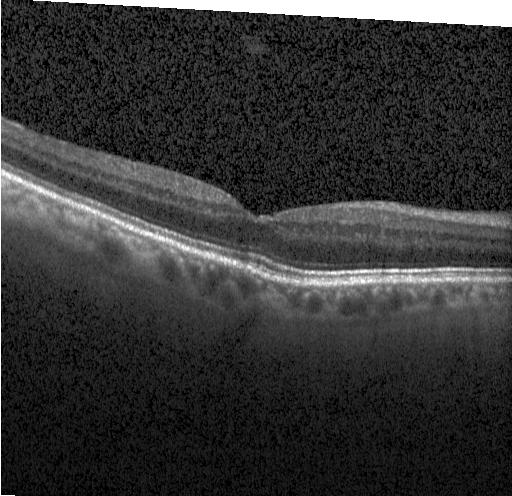

Instrument: Heidelberg Spectralis. Retinal OCT cross-section. Macular scan. This B-scan demonstrates neither CNV, DME, nor drusen.